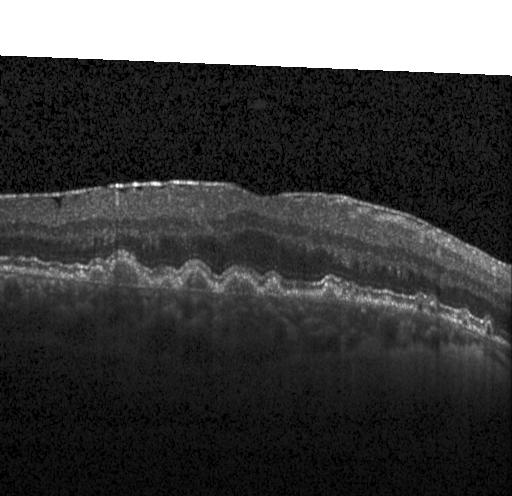

Retinal OCT cross-section; centered on the fovea. Finding: drusen.